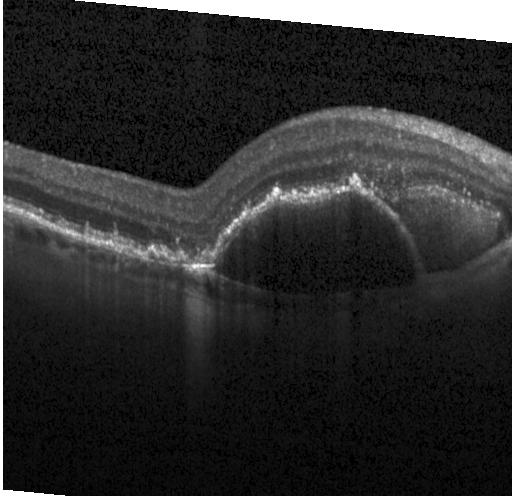
Macular OCT: a choroidal neovascular membrane.